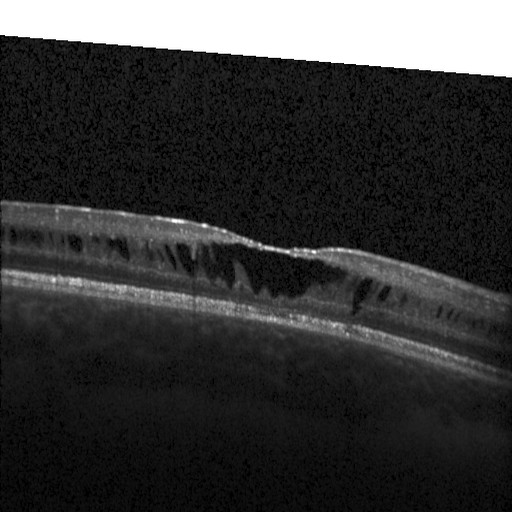

The scan shows DME.